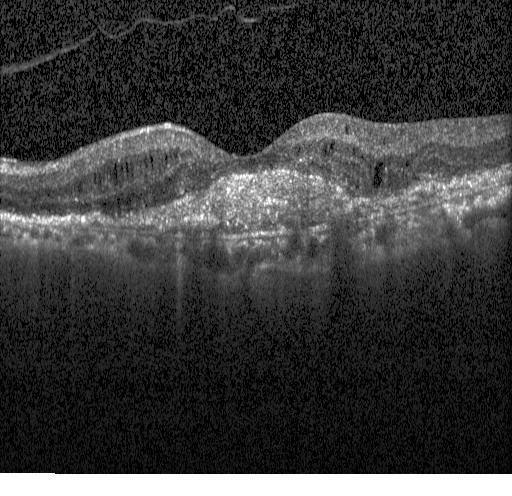
Horizontal scan through the fovea · retinal OCT cross-section.
Dx: a choroidal neovascular membrane.